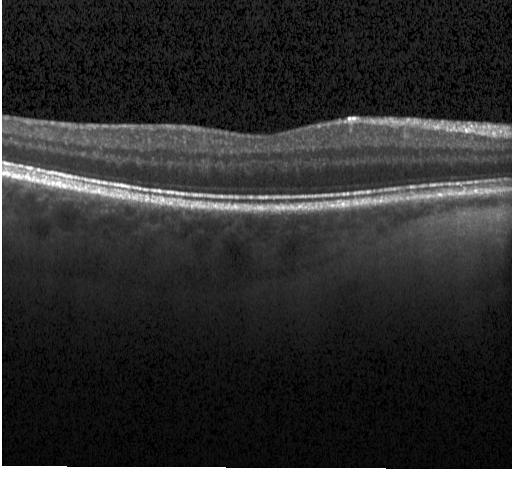 Optical coherence tomography B-scan, Heidelberg Spectralis OCT system — No CNV, no DME, and no drusen.